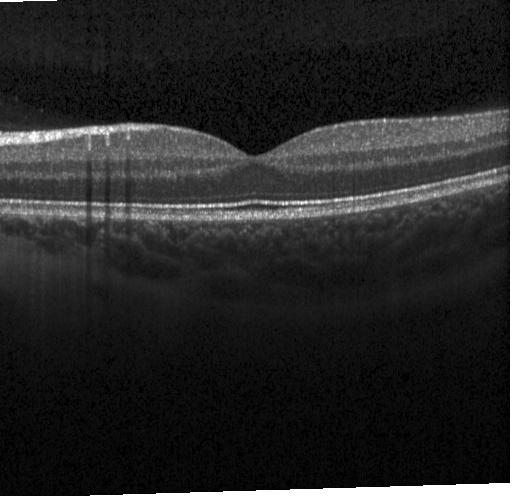 Dx: no evidence of choroidal neovascularization, diabetic macular edema, or drusen.